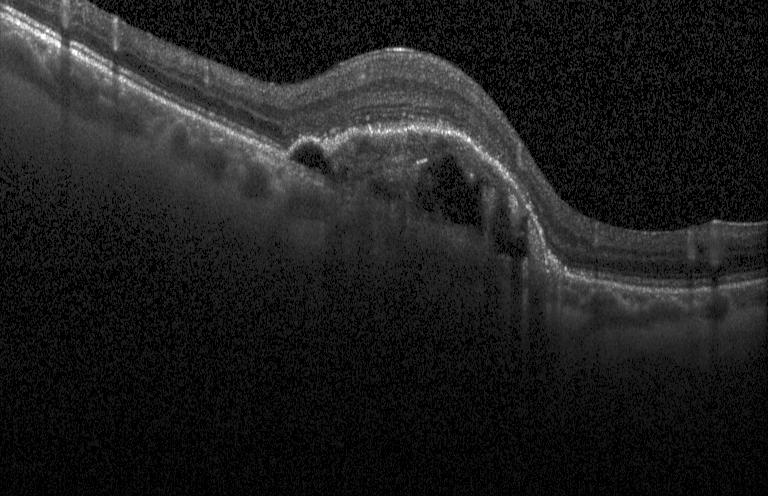
A choroidal neovascular membrane.